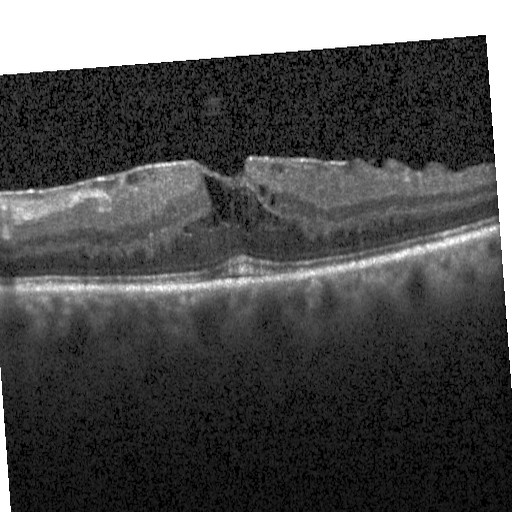 OCT scan showing DME.